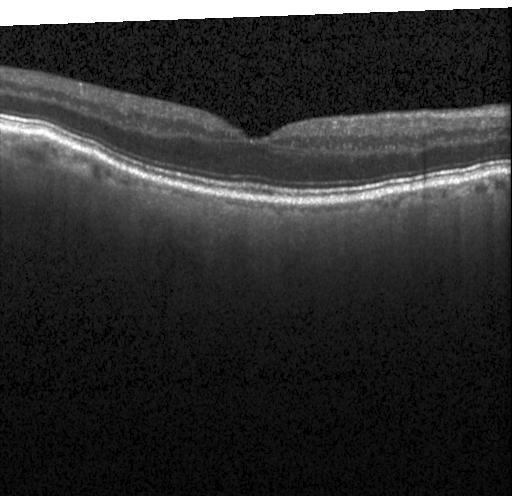
The scan shows no evidence of CNV, DME, or drusen.